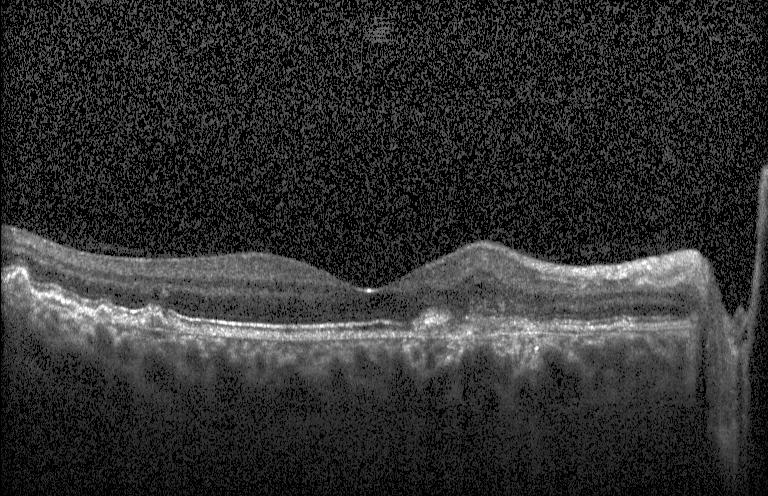

SD-OCT · acquired on a Heidelberg Spectralis · optical coherence tomography B-scan · through the macula.
Impression: a choroidal neovascular membrane.